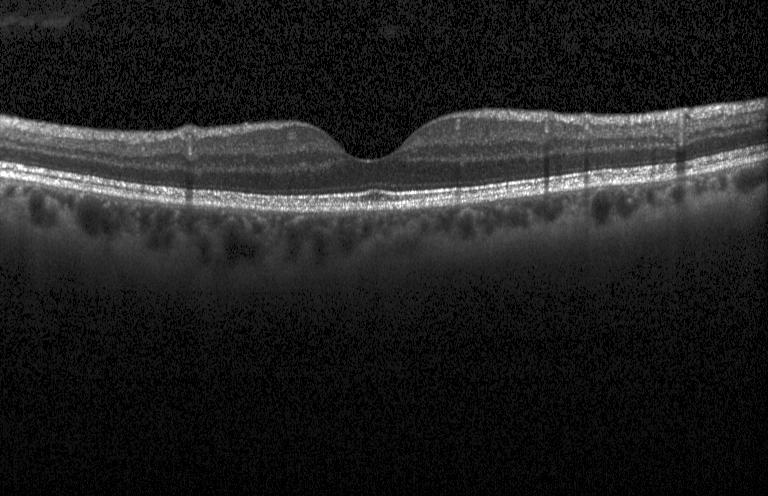 Acquired on a Heidelberg Spectralis; OCT line scan. Impression: neither choroidal neovascularization, diabetic macular edema, nor drusen.